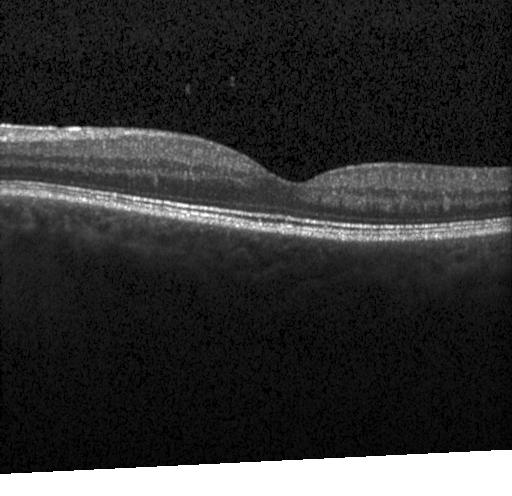

Heidelberg Spectralis, optical coherence tomography scan, centered on the fovea
Impression: neither CNV, DME, nor drusen.